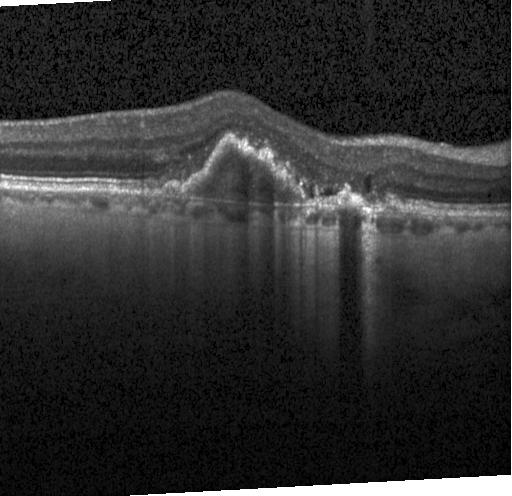
OCT B-scan; horizontal scan through the fovea.
Dx: choroidal neovascularization.